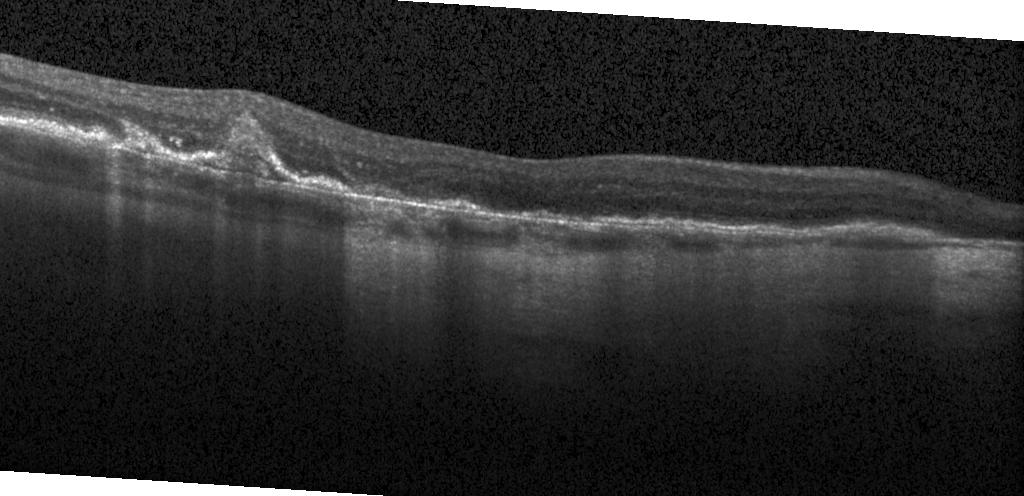 Centered on the fovea · retinal OCT B-scan · spectral-domain optical coherence tomography · instrument: Heidelberg Spectralis.
Impression: a choroidal neovascular membrane.